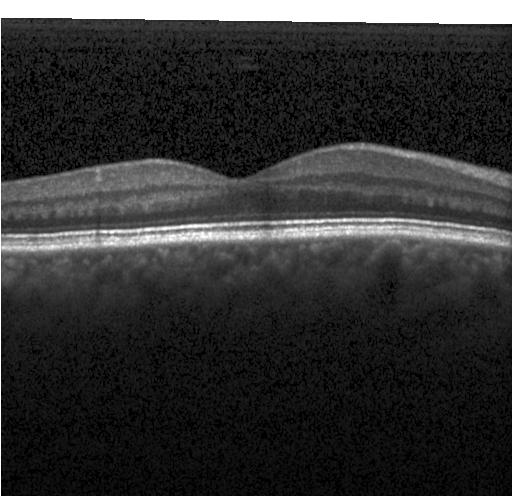

Dx: neither choroidal neovascularization, diabetic macular edema, nor drusen.